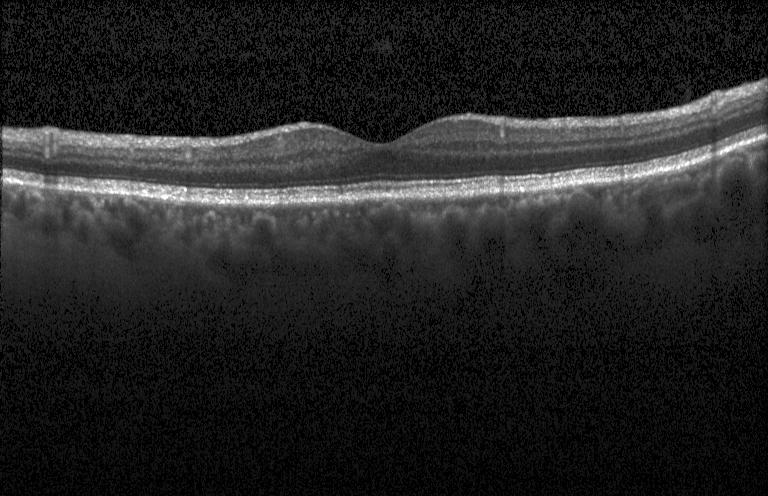
Instrument: Heidelberg Spectralis. OCT line scan. Spectral-domain optical coherence tomography
No CNV, DME, or drusen.